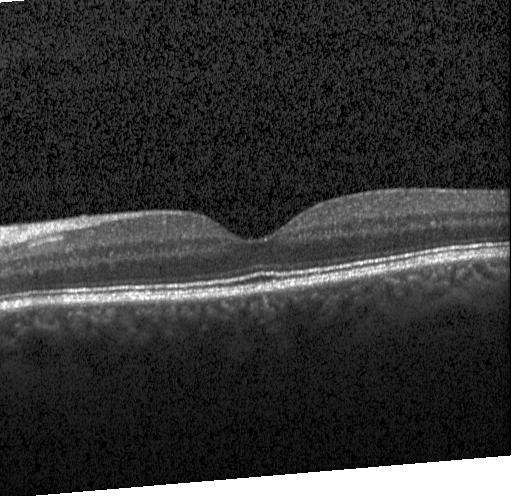

Heidelberg Spectralis OCT system · retinal OCT cross-section · through the macula — This B-scan demonstrates no CNV, no DME, and no drusen.